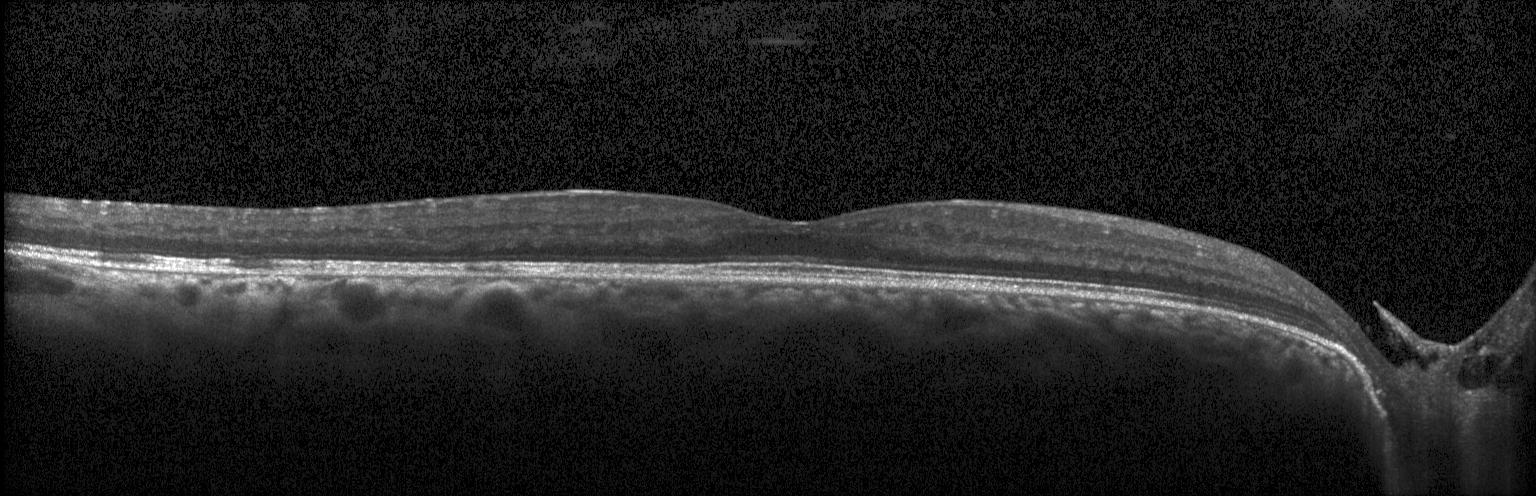

Macular scan, SD-OCT, optical coherence tomography B-scan, Heidelberg Spectralis. Impression: no CNV, DME, or drusen.